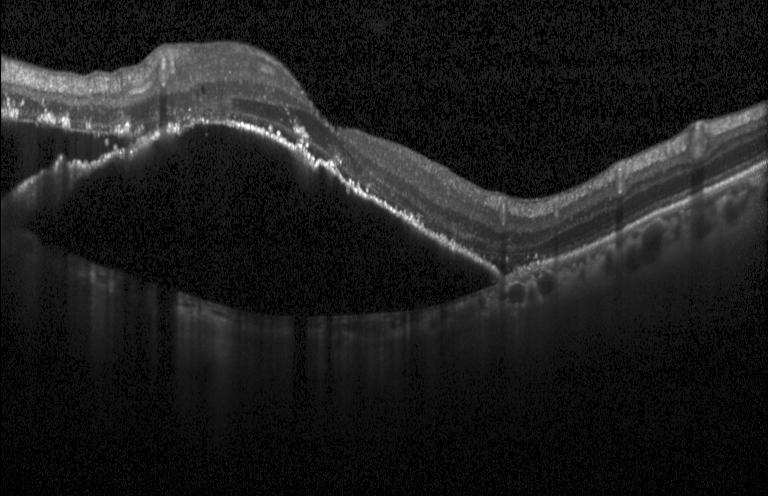

OCT line scan — Assessment: a choroidal neovascular membrane.